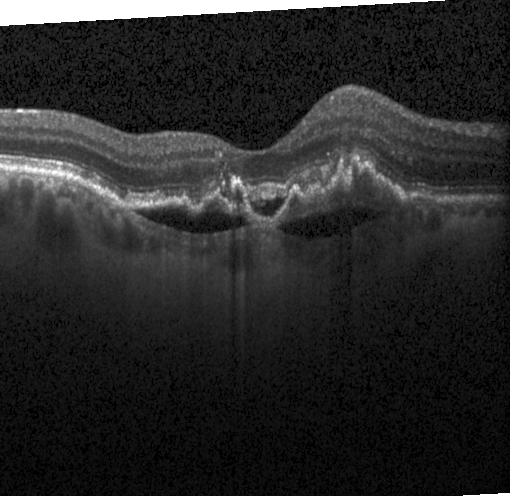 Finding: choroidal neovascularization.